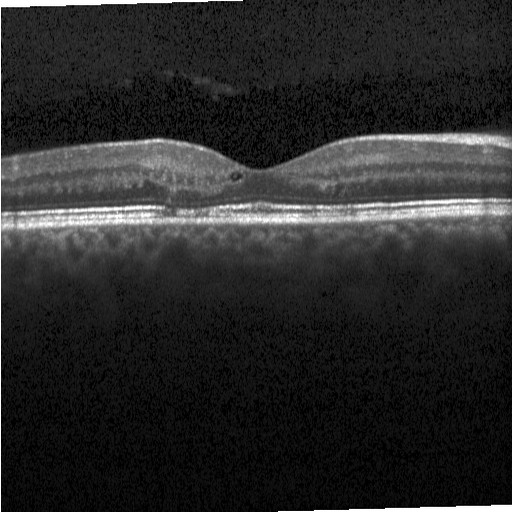
Assessment: diabetic macular edema.